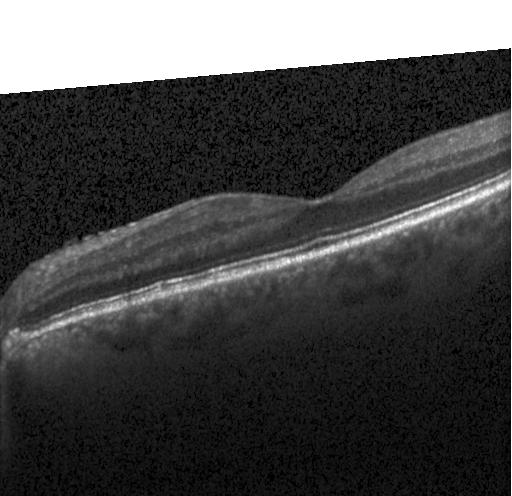

Optical coherence tomography B-scan; Heidelberg Spectralis
No evidence of choroidal neovascularization, diabetic macular edema, or drusen.